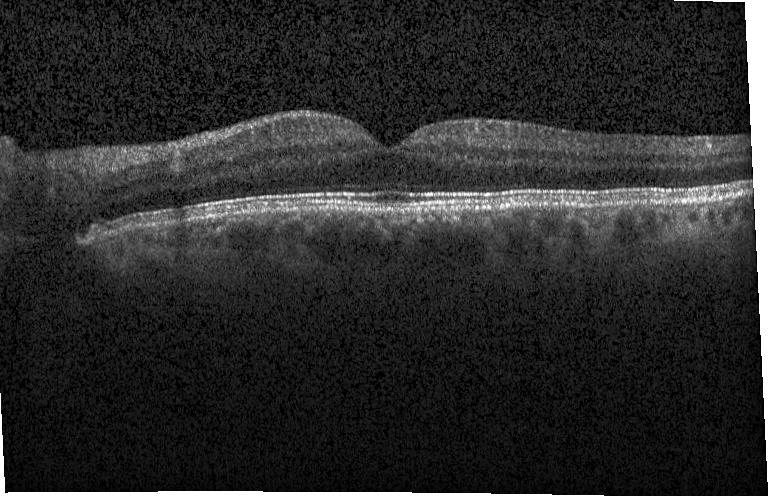

This B-scan demonstrates no CNV, DME, or drusen.